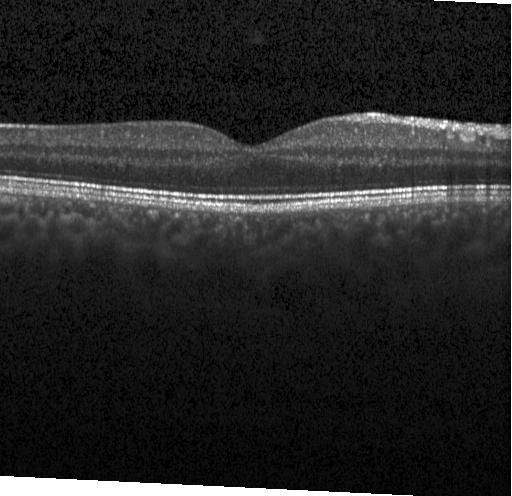
Retinal OCT B-scan.
Impression: no evidence of CNV, DME, or drusen.